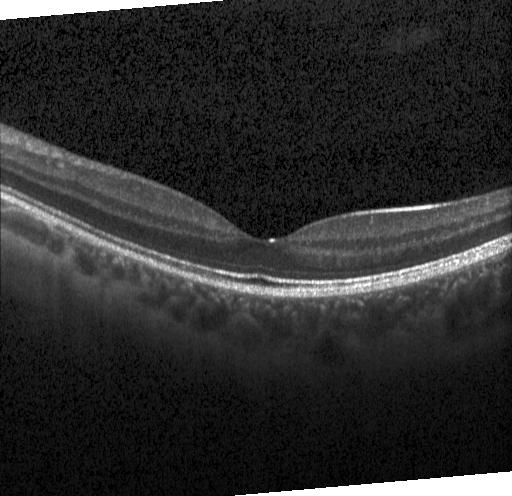
Macular scan, Heidelberg Spectralis, SD-OCT, retinal OCT B-scan.
Impression: no choroidal neovascularization, no diabetic macular edema, and no drusen.